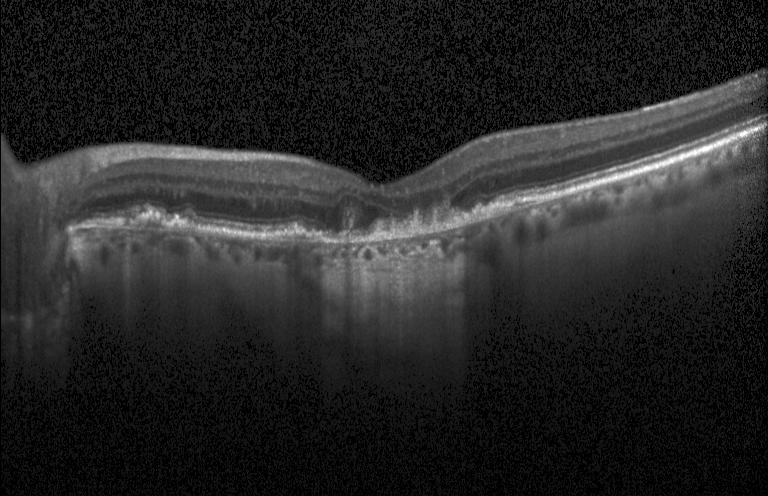
Macular OCT: choroidal neovascularization (CNV).